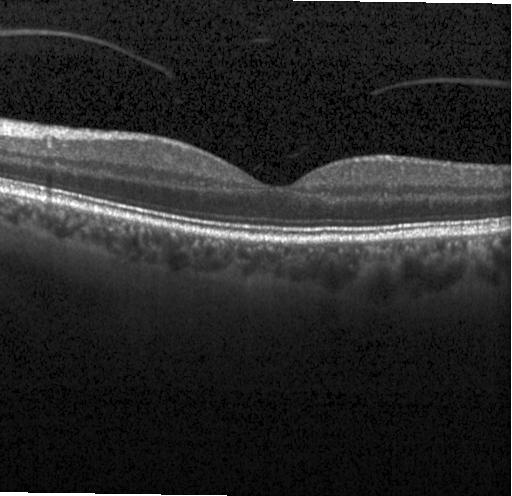 OCT B-scan, spectral-domain optical coherence tomography. OCT finding: neither CNV, DME, nor drusen.